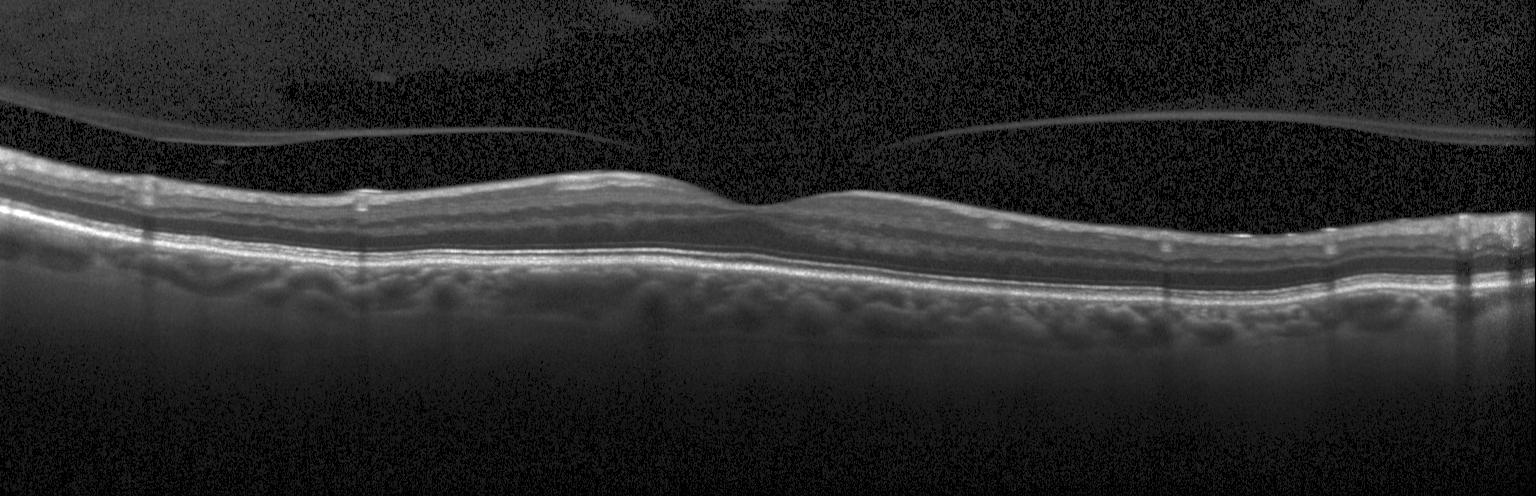
Diagnosis: no evidence of CNV, DME, or drusen.